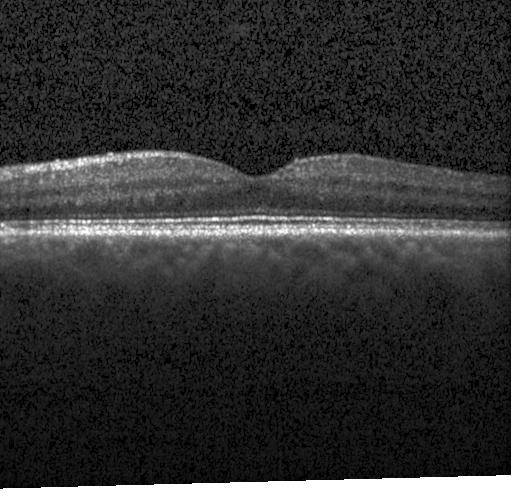 Diagnosis: no CNV, DME, or drusen.